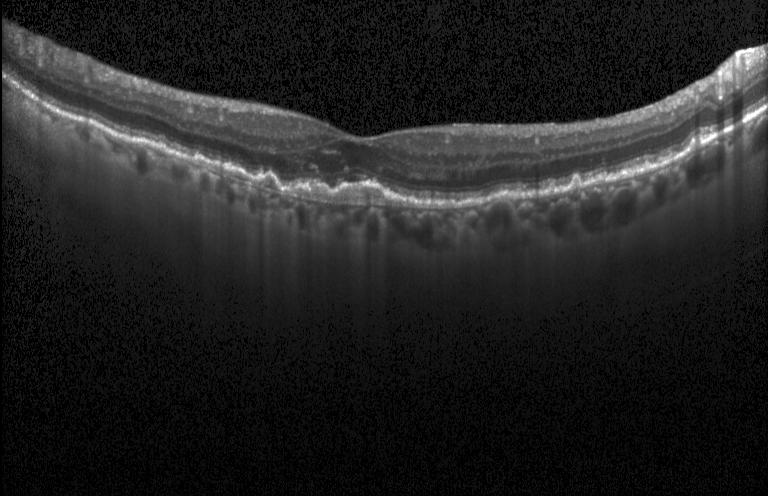
Dx: a choroidal neovascular membrane.